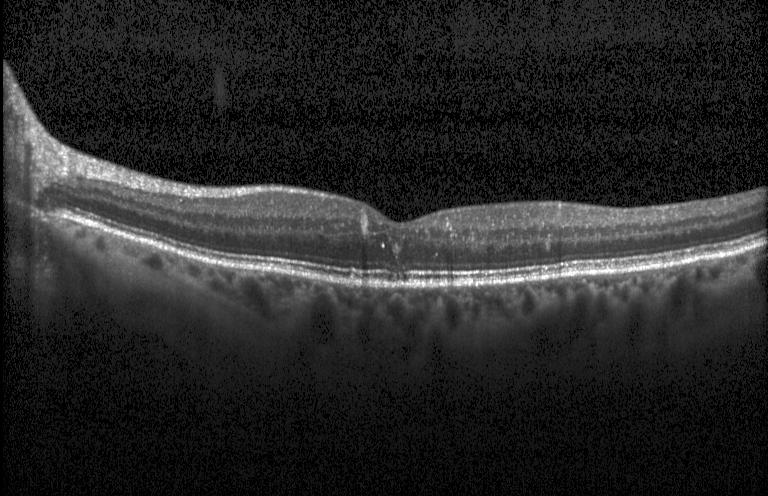 Diagnosis: no choroidal neovascularization, diabetic macular edema, or drusen.